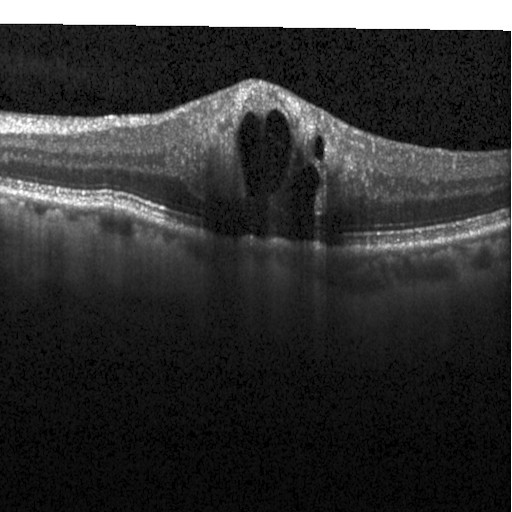 DME.